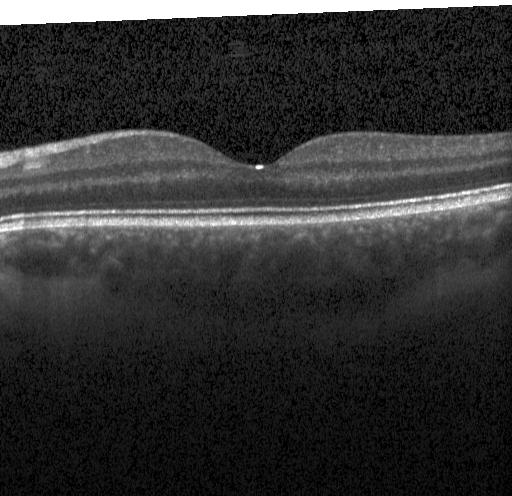

Instrument: Heidelberg Spectralis · spectral-domain optical coherence tomography · optical coherence tomography B-scan. Impression: neither choroidal neovascularization, diabetic macular edema, nor drusen.